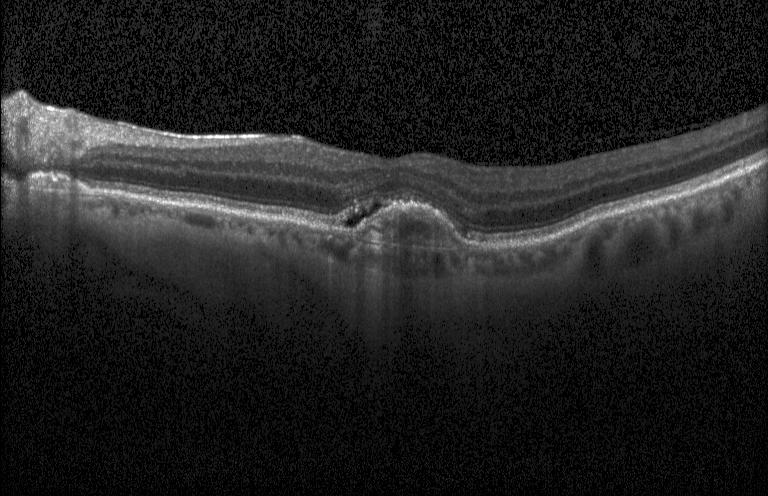
Instrument: Heidelberg Spectralis · spectral-domain optical coherence tomography · centered on the fovea · optical coherence tomography B-scan.
Impression: a choroidal neovascular membrane.